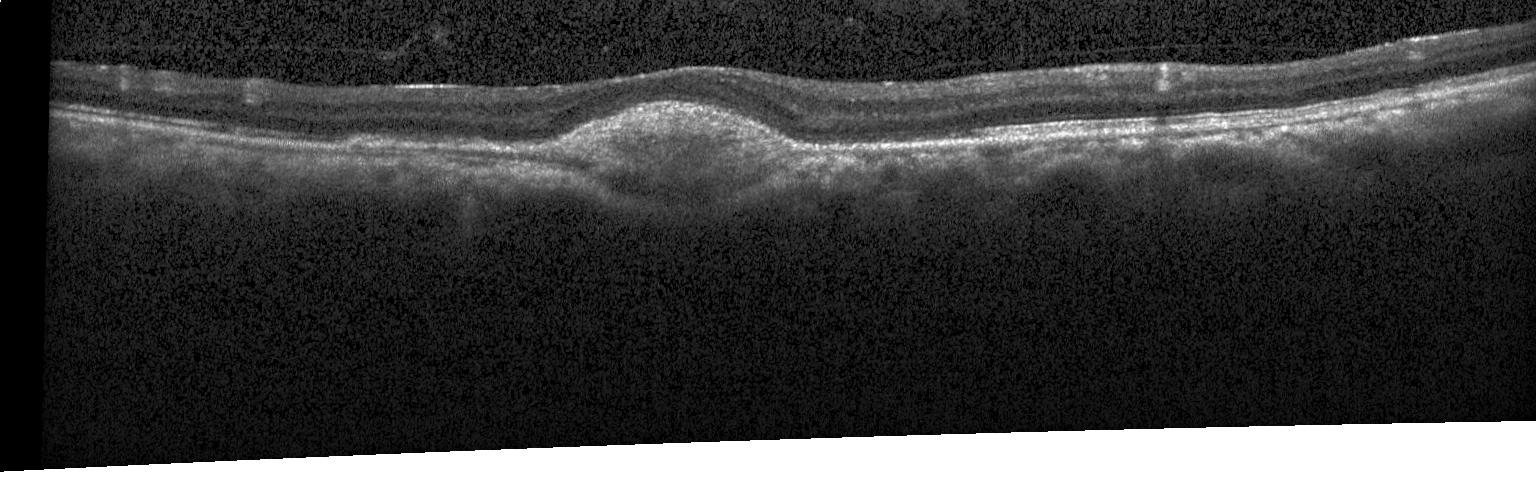

OCT line scan · acquired on a Heidelberg Spectralis · fovea-centered · spectral-domain OCT — Assessment: choroidal neovascularization.